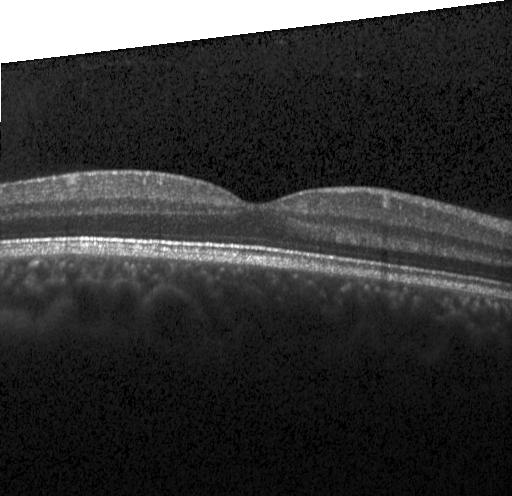
Acquired on a Heidelberg Spectralis · horizontal scan through the fovea · OCT line scan — Diagnosis: no CNV, DME, or drusen.